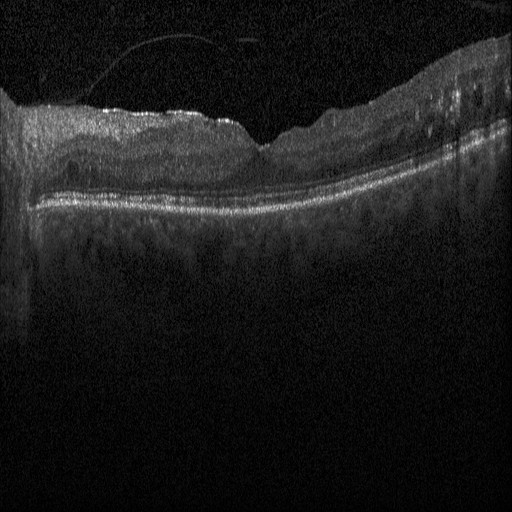 SD-OCT · OCT line scan · horizontal scan through the fovea
Diagnosis: DME.